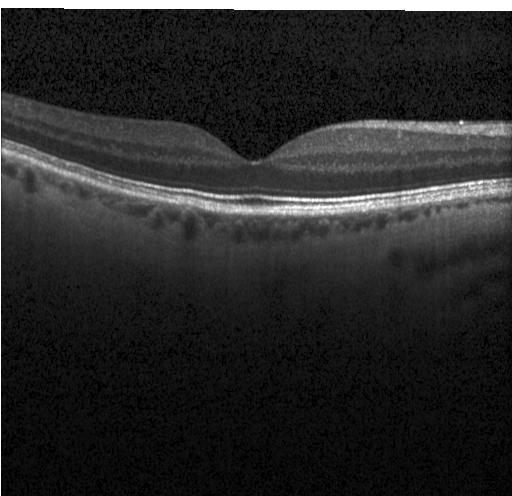

Diagnosis: no evidence of choroidal neovascularization, diabetic macular edema, or drusen.